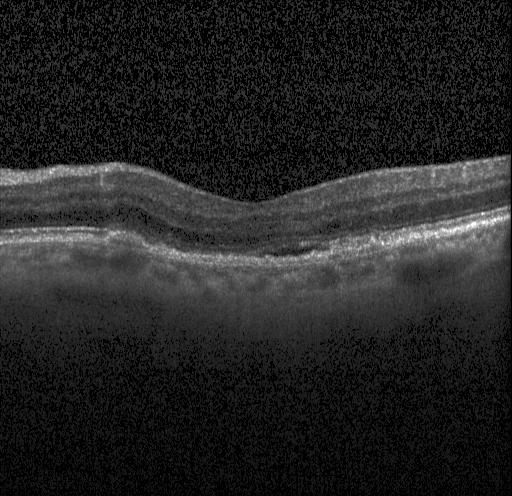
Heidelberg Spectralis · retinal OCT cross-section · horizontal scan through the fovea
This B-scan demonstrates choroidal neovascularization.